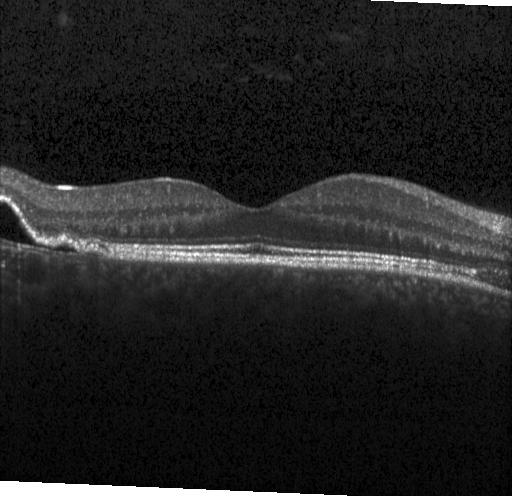
OCT B-scan; SD-OCT; through the macula — Finding: a choroidal neovascular membrane.